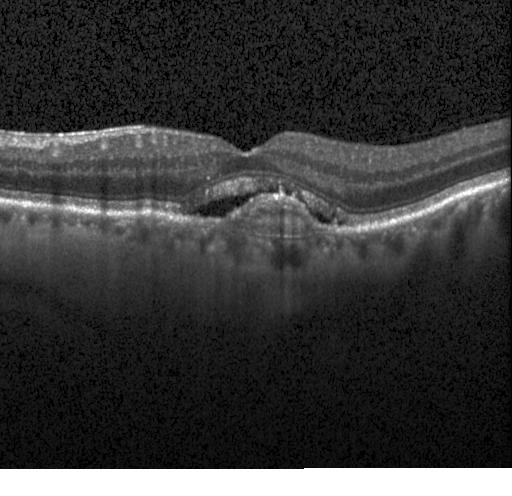

Instrument: Heidelberg Spectralis; horizontal scan through the fovea; optical coherence tomography scan — The scan shows choroidal neovascularization.